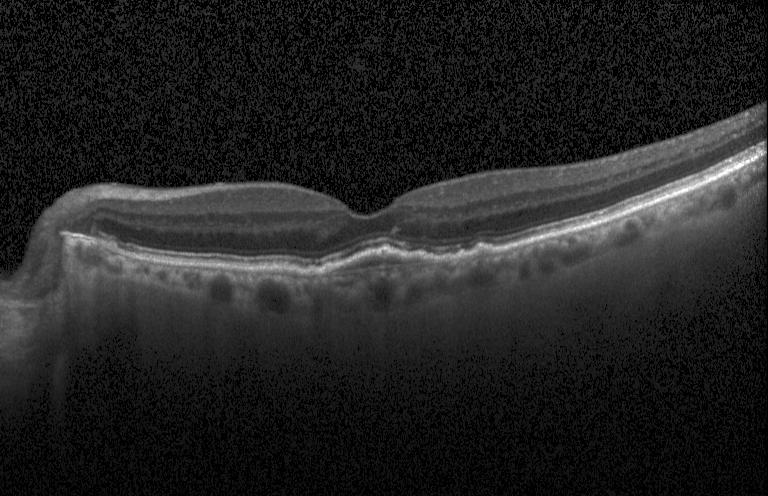 Instrument: Heidelberg Spectralis; spectral-domain OCT; optical coherence tomography scan.
Impression: CNV.